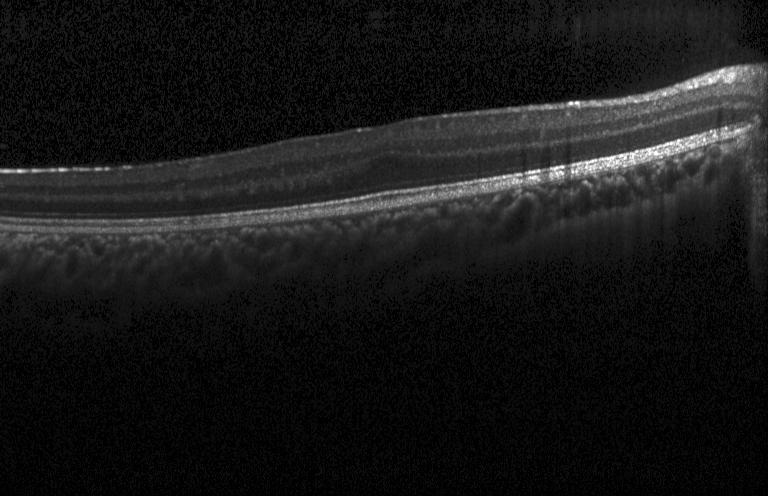

Spectral-domain optical coherence tomography · retinal OCT B-scan · centered on the fovea
Assessment: no CNV, DME, or drusen.